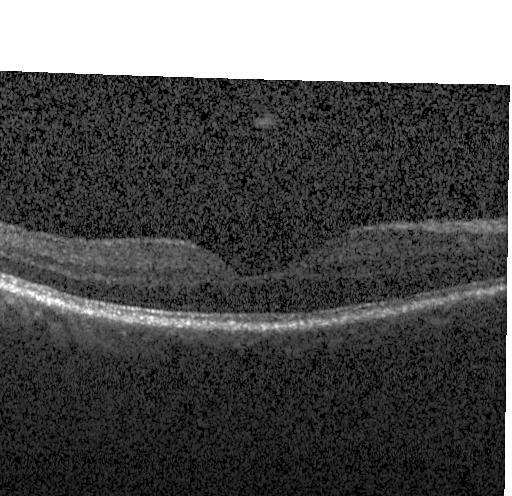 OCT B-scan — This B-scan demonstrates no choroidal neovascularization, diabetic macular edema, or drusen.